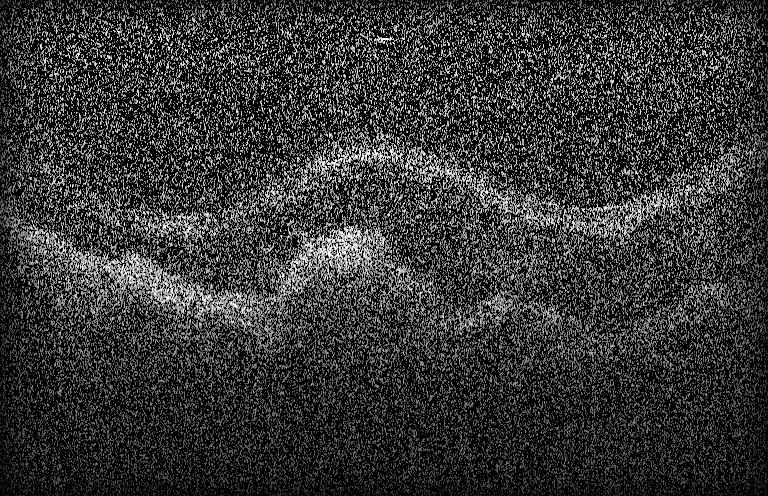
Finding: choroidal neovascularization.